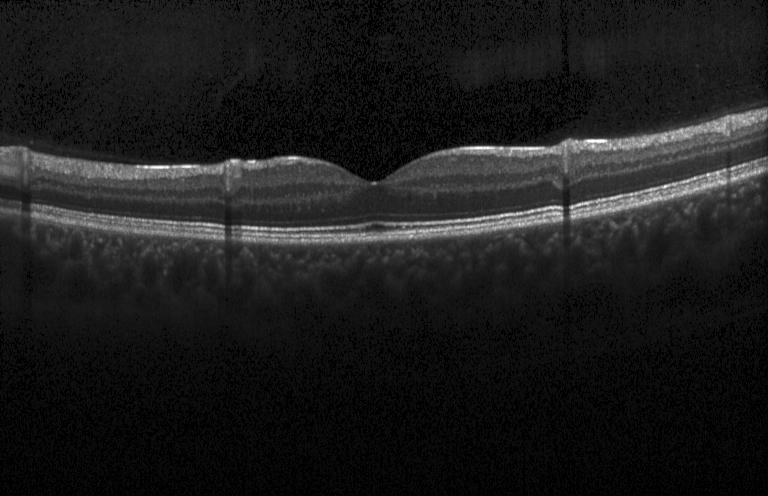

Diagnosis: no evidence of choroidal neovascularization, diabetic macular edema, or drusen.